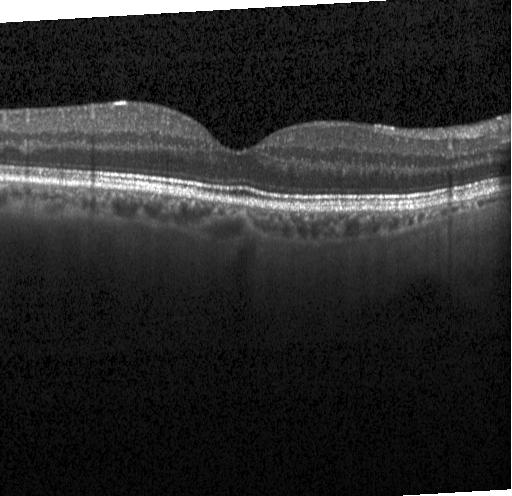
Diagnosis: no choroidal neovascularization, diabetic macular edema, or drusen.